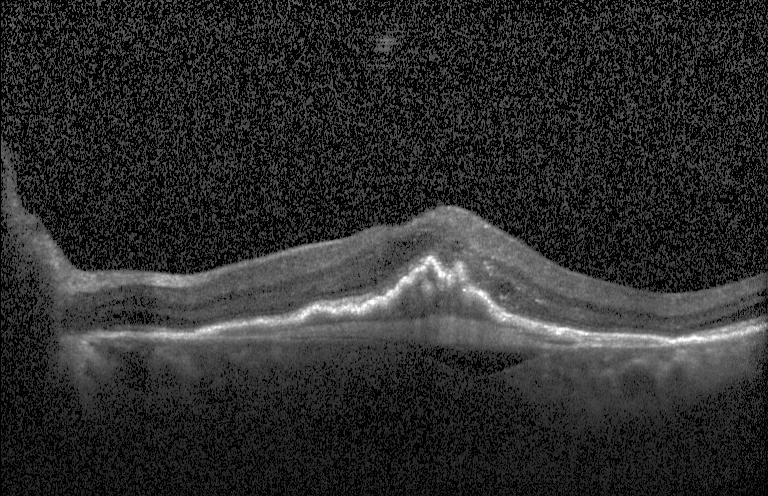

Optical coherence tomography B-scan; spectral-domain optical coherence tomography; Heidelberg Spectralis OCT system — Assessment: a choroidal neovascular membrane.